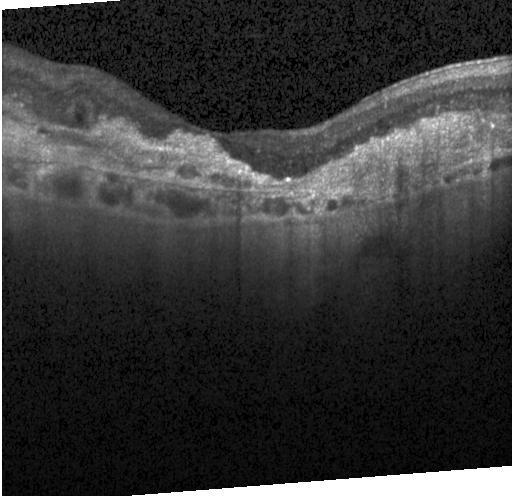

Diagnosis: a choroidal neovascular membrane.